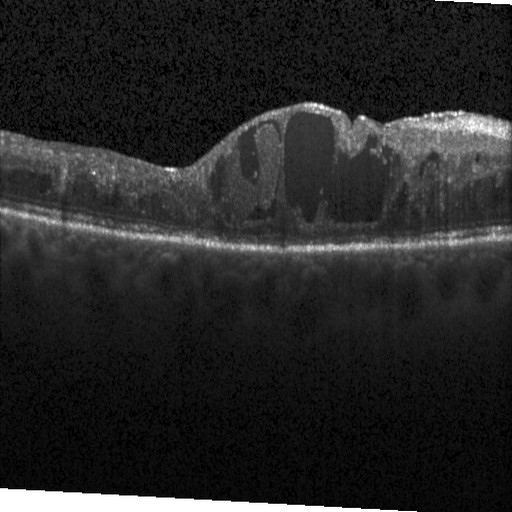

Spectral-domain OCT; OCT B-scan; fovea-centered; Heidelberg Spectralis.
Diagnosis: diabetic macular edema.